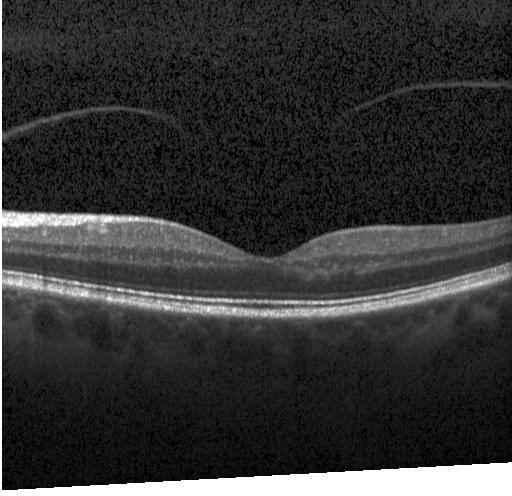

OCT scan showing no CNV, no DME, and no drusen.